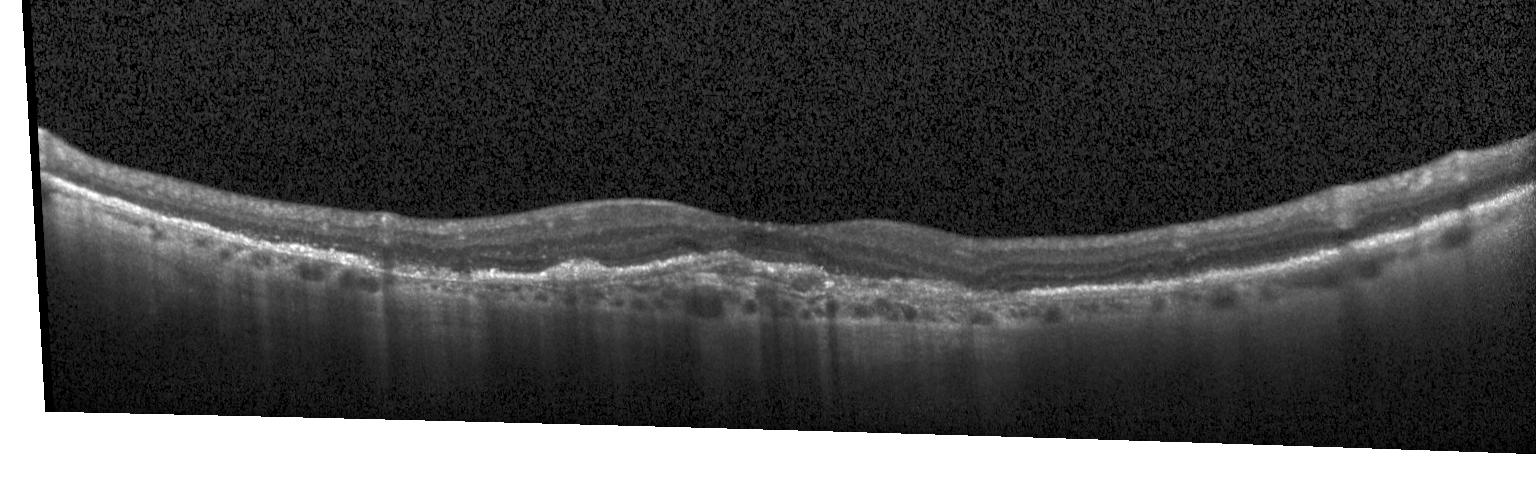

Finding: choroidal neovascularization.